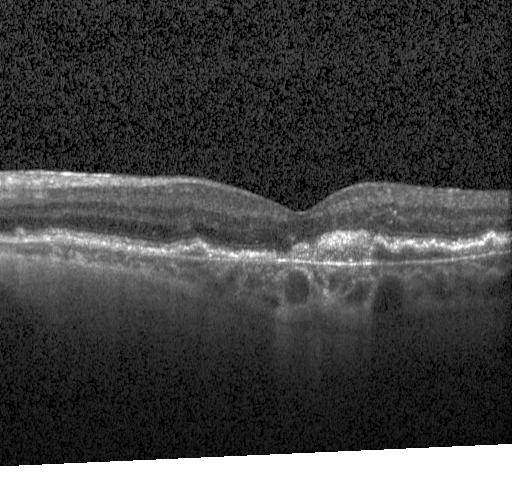
Assessment: choroidal neovascularization.